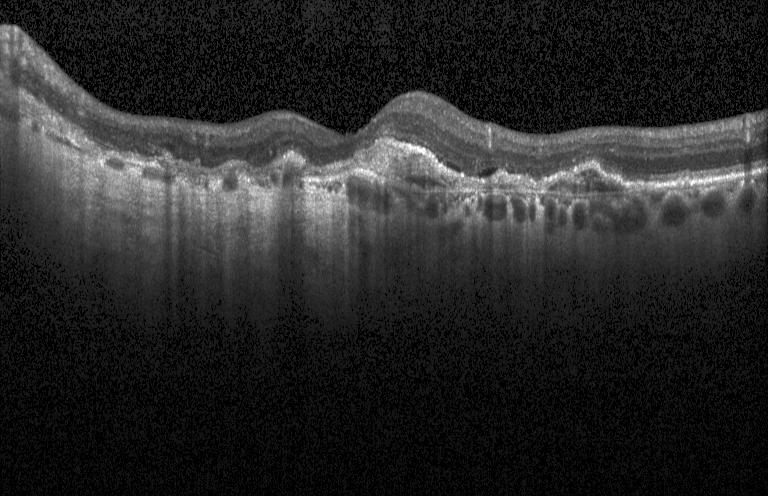 A choroidal neovascular membrane.